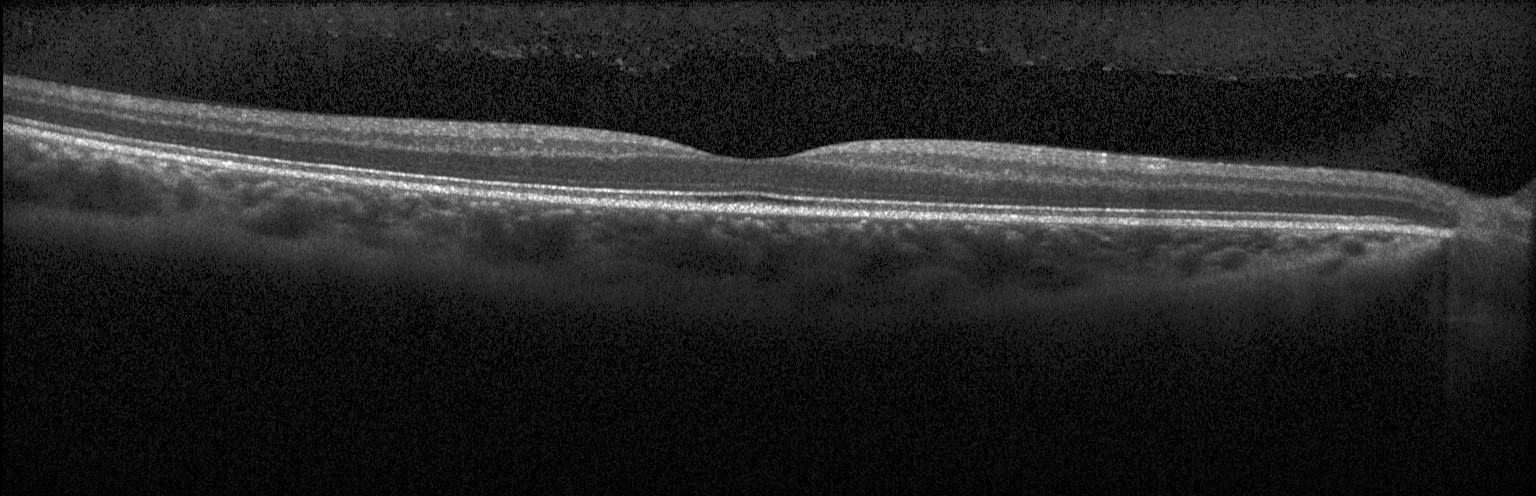
OCT finding: no choroidal neovascularization, no diabetic macular edema, and no drusen.